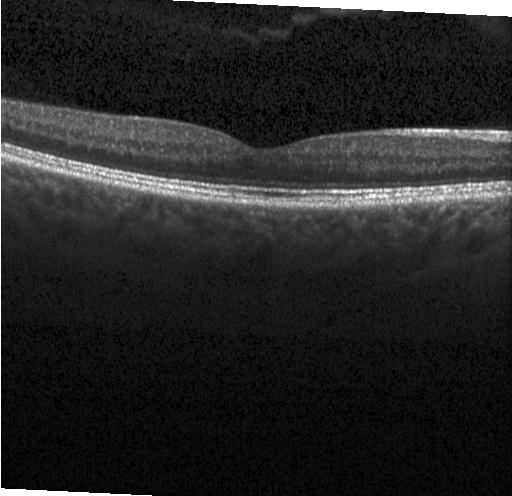
Macular scan. Heidelberg Spectralis. OCT B-scan. SD-OCT. Diagnosis: no evidence of choroidal neovascularization, diabetic macular edema, or drusen.